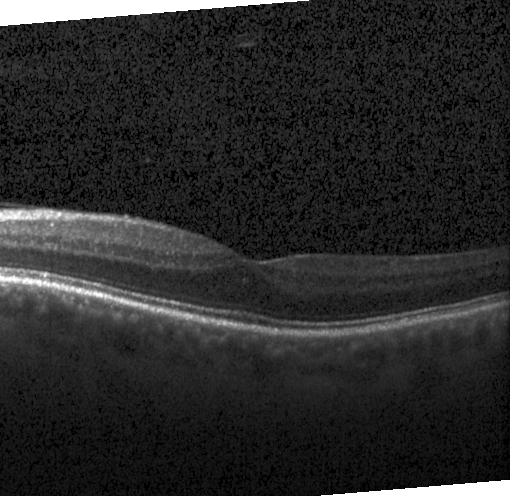

Assessment: no evidence of choroidal neovascularization, diabetic macular edema, or drusen.